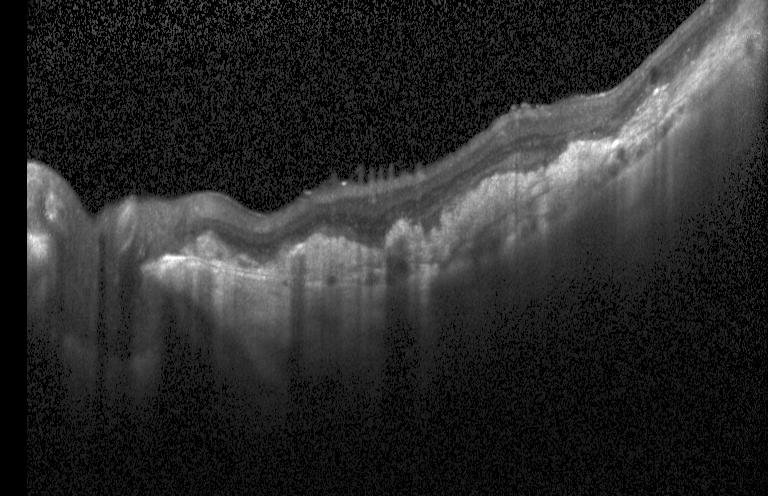 This B-scan demonstrates a choroidal neovascular membrane.